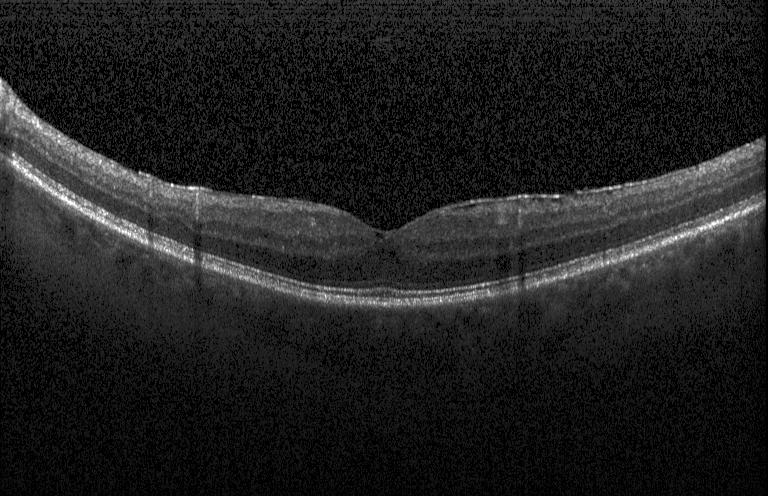
OCT scan showing no choroidal neovascularization, no diabetic macular edema, and no drusen.